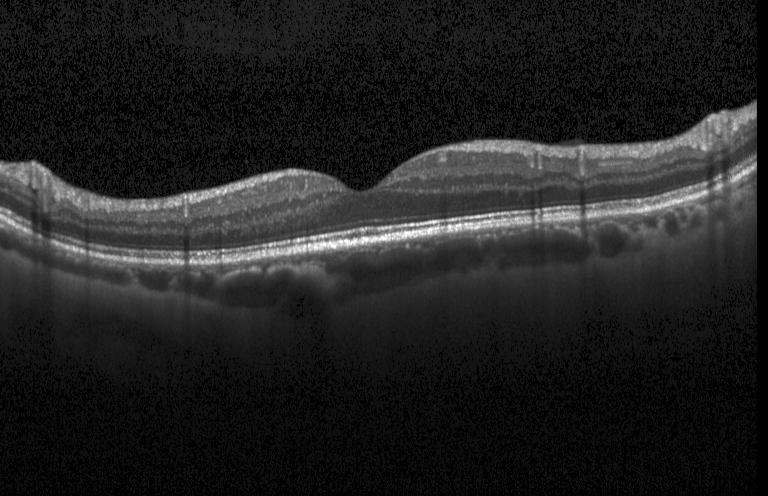 SD-OCT. Acquired on a Heidelberg Spectralis. OCT B-scan. Macular scan. This B-scan demonstrates no CNV, DME, or drusen.